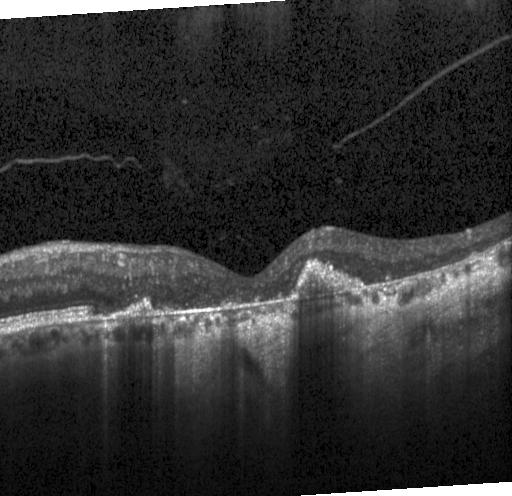
OCT scan showing a choroidal neovascular membrane.